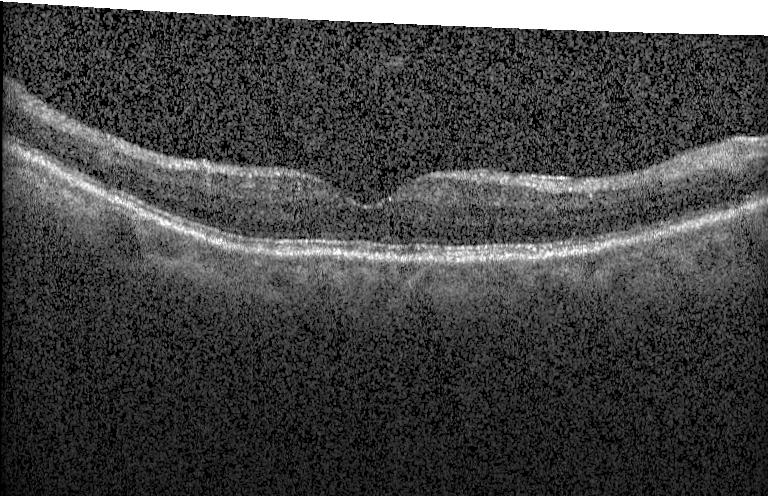 OCT line scan, acquired on a Heidelberg Spectralis, SD-OCT.
Diagnosis: neither choroidal neovascularization, diabetic macular edema, nor drusen.